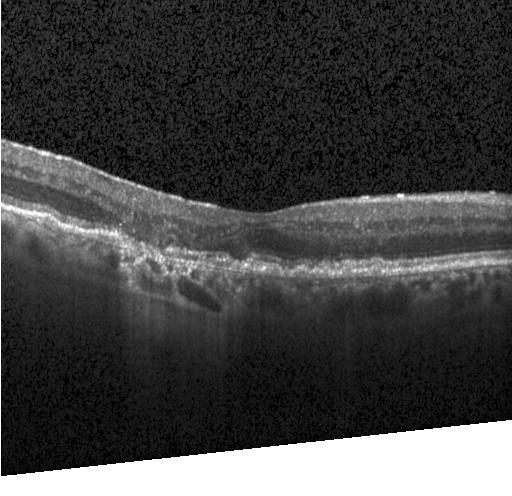

Macular scan · spectral-domain OCT · retinal OCT cross-section — Finding: CNV.